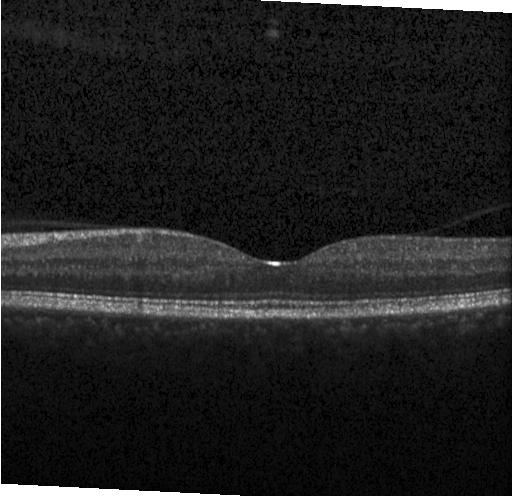

Spectral-domain optical coherence tomography; retinal OCT cross-section
Impression: no choroidal neovascularization, no diabetic macular edema, and no drusen.